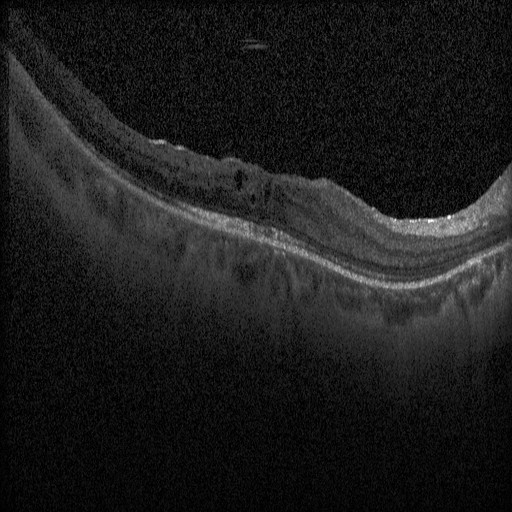 OCT B-scan. Diagnosis: DME.